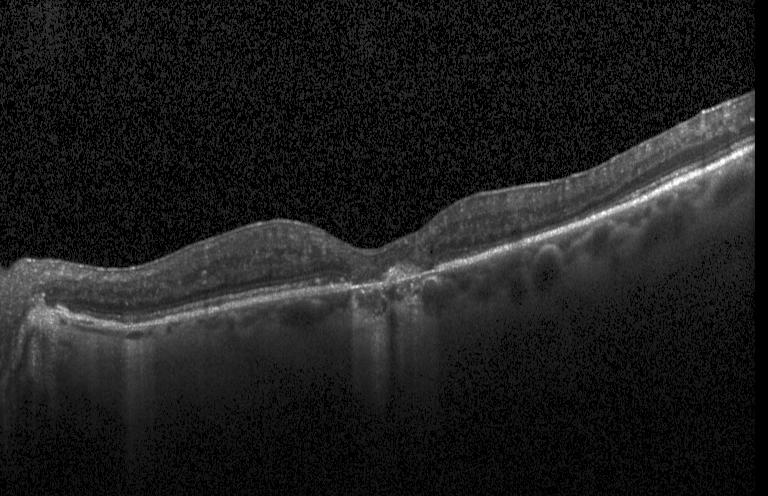 Finding: a choroidal neovascular membrane.